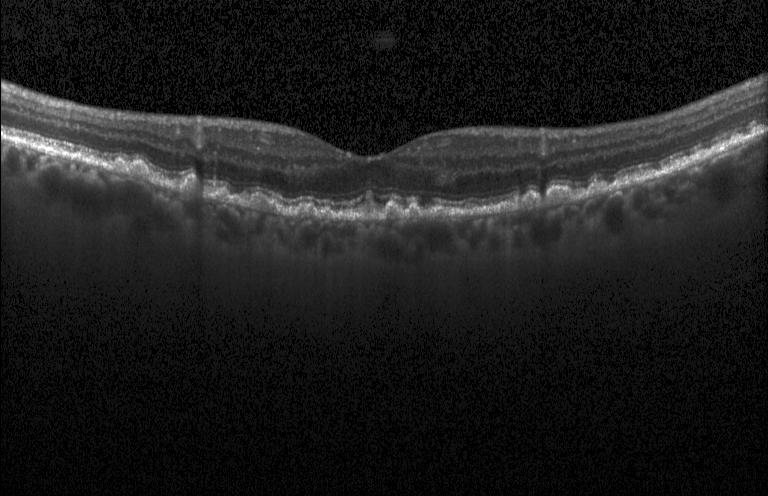 Retinal OCT cross-section.
Diagnosis: sub-RPE drusenoid deposits.